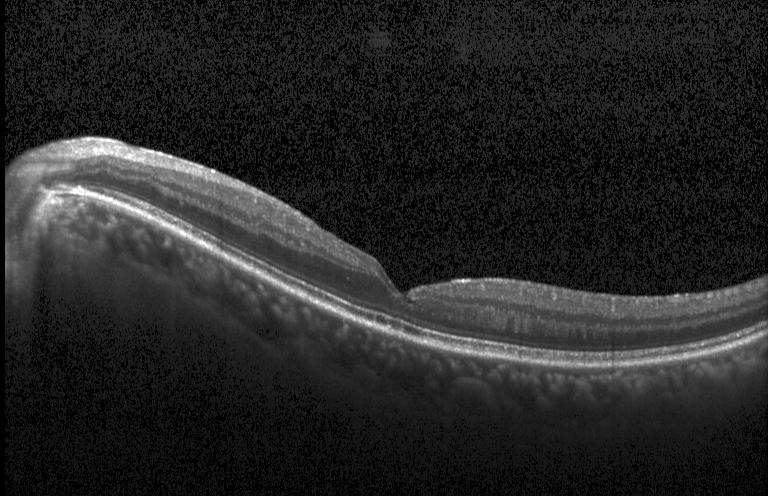

Macular OCT: no choroidal neovascularization, diabetic macular edema, or drusen.